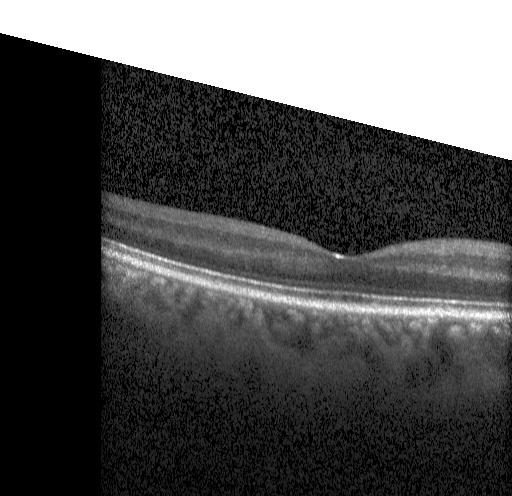

Optical coherence tomography B-scan
Macular OCT: no evidence of choroidal neovascularization, diabetic macular edema, or drusen.